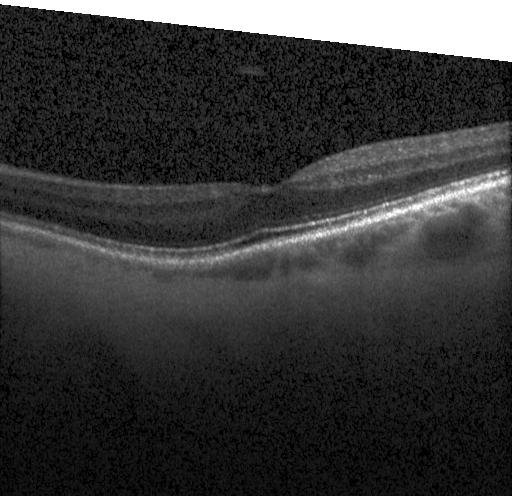
OCT line scan, SD-OCT, Heidelberg Spectralis, fovea-centered.
Dx: no choroidal neovascularization, diabetic macular edema, or drusen.